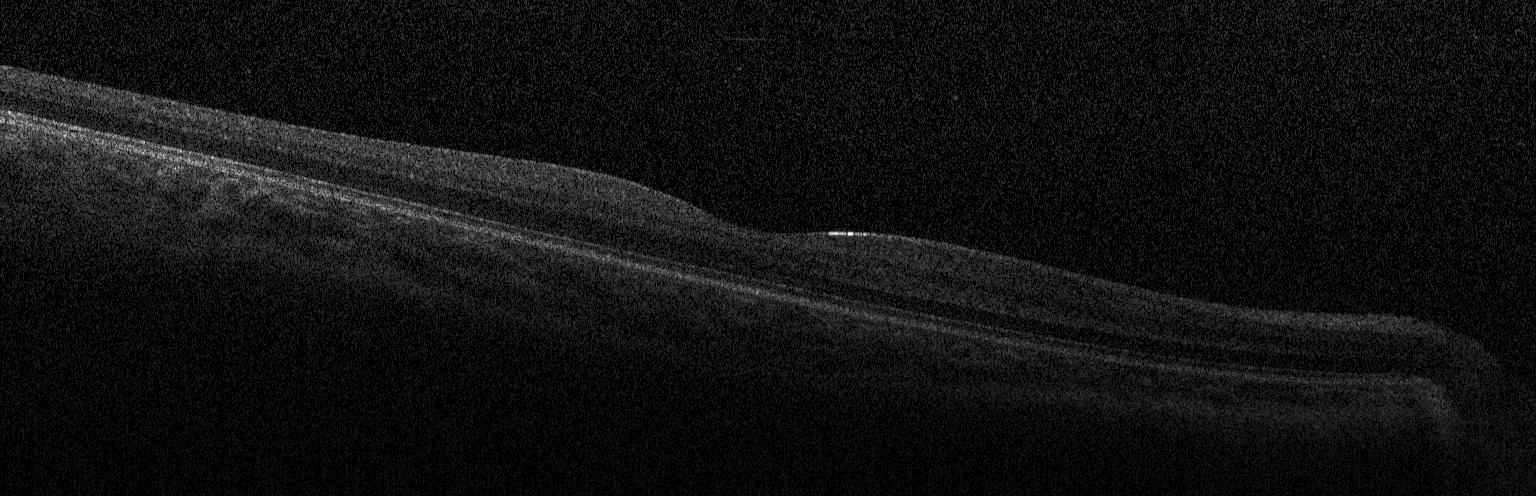 Retinal OCT cross-section showing no evidence of choroidal neovascularization, diabetic macular edema, or drusen.